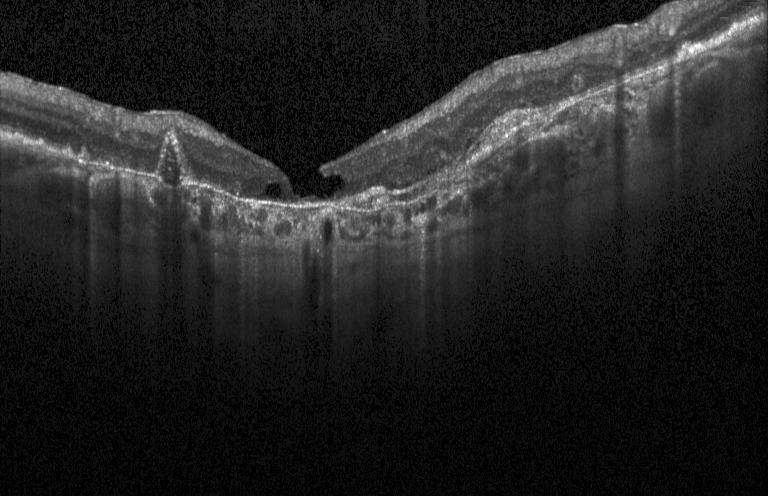

Horizontal scan through the fovea · spectral-domain optical coherence tomography · OCT line scan.
Impression: choroidal neovascularization (CNV).